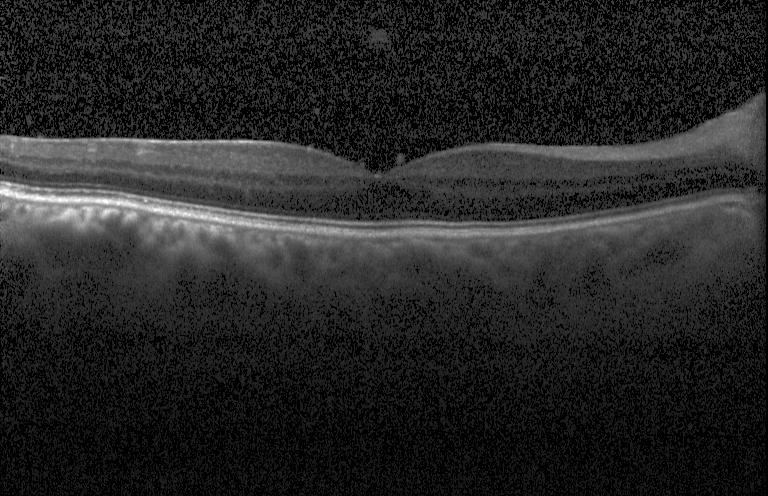
Optical coherence tomography scan — This B-scan demonstrates no choroidal neovascularization, no diabetic macular edema, and no drusen.